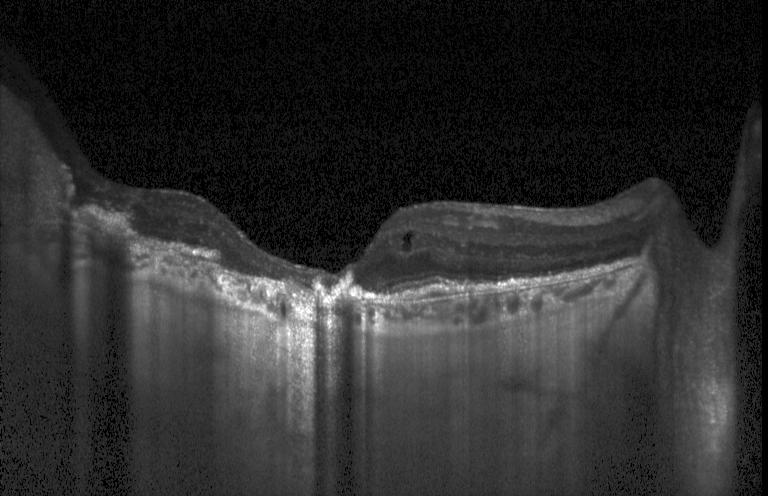 Retinal OCT B-scan — Impression: a choroidal neovascular membrane.